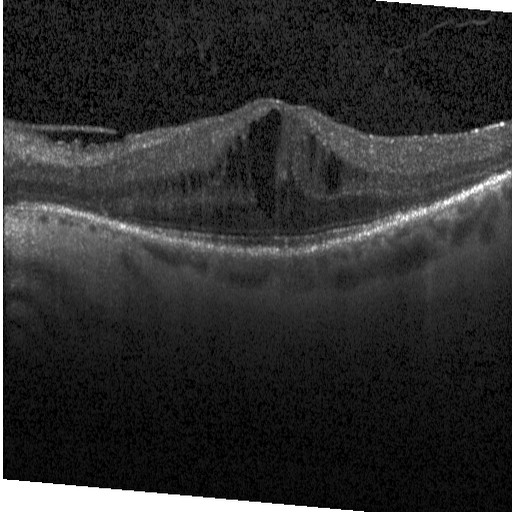
OCT scan showing diabetic macular edema (DME).